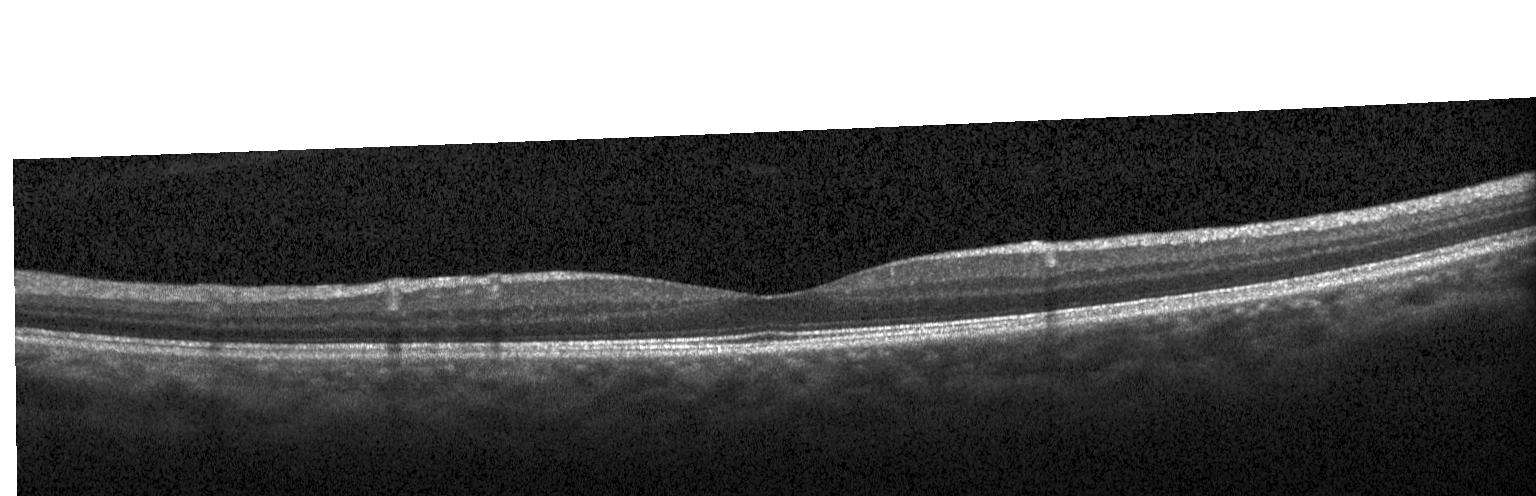 SD-OCT. Retinal OCT B-scan. Acquired on a Heidelberg Spectralis. Horizontal scan through the fovea. Impression: no evidence of choroidal neovascularization, diabetic macular edema, or drusen.